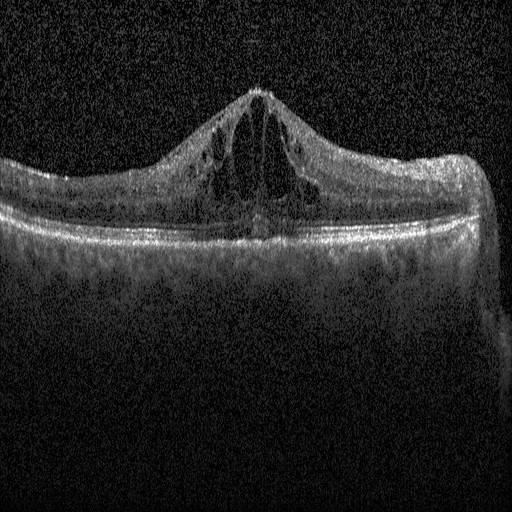
Impression: diabetic macular edema.